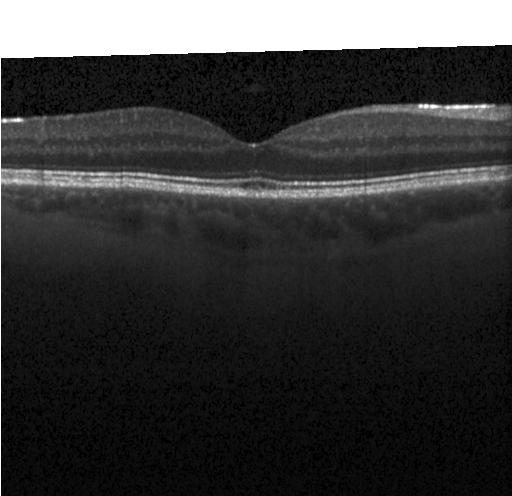
Finding: neither choroidal neovascularization, diabetic macular edema, nor drusen.